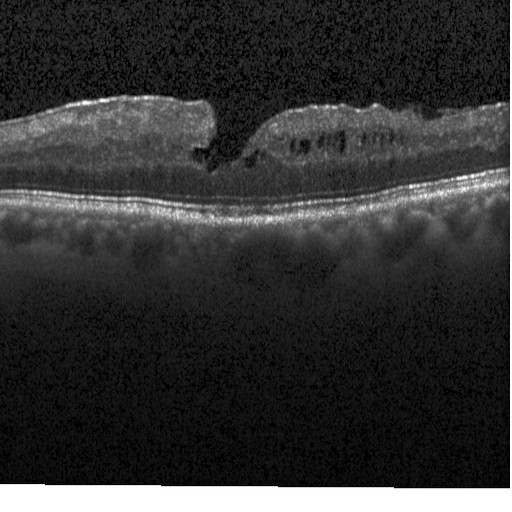
The scan shows diabetic macular edema.